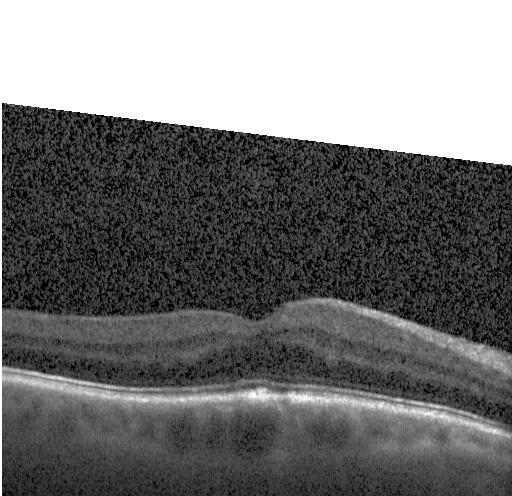

Retinal OCT cross-section — Finding: no evidence of choroidal neovascularization, diabetic macular edema, or drusen.